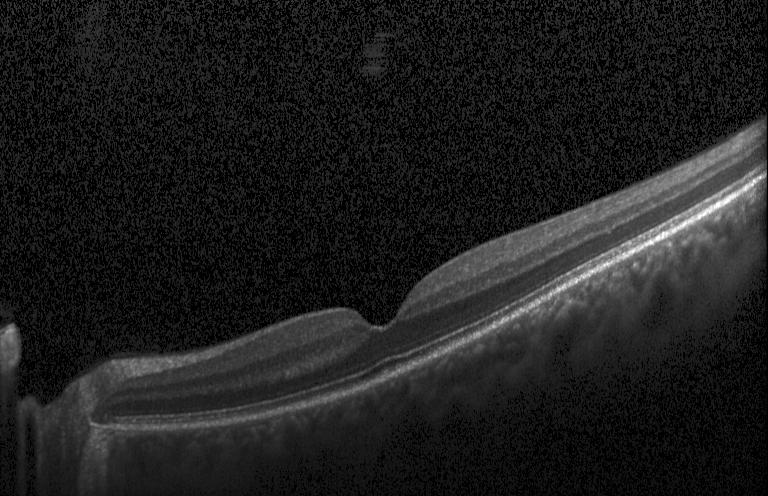 Macular OCT demonstrating no evidence of CNV, DME, or drusen.